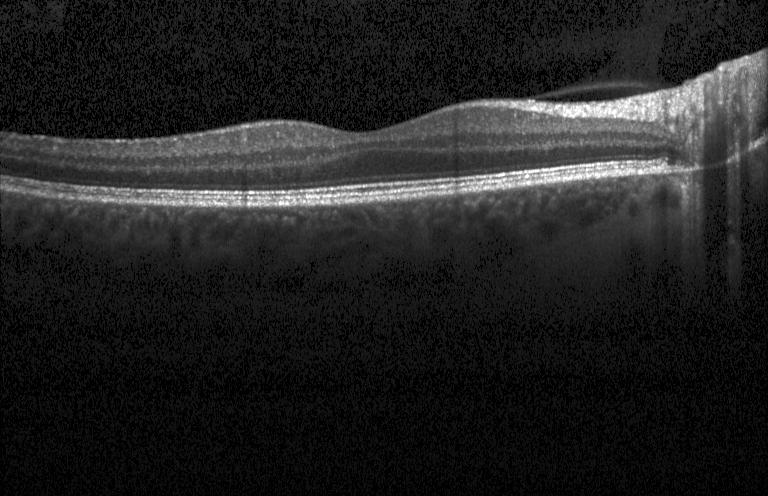

OCT B-scan — Dx: no choroidal neovascularization, no diabetic macular edema, and no drusen.